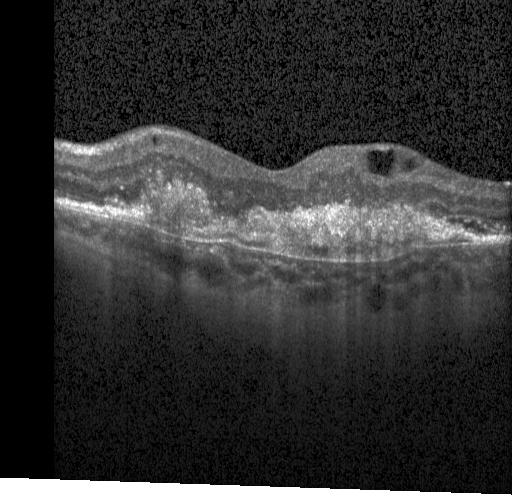

Optical coherence tomography scan. Through the macula. Diagnosis: a choroidal neovascular membrane.